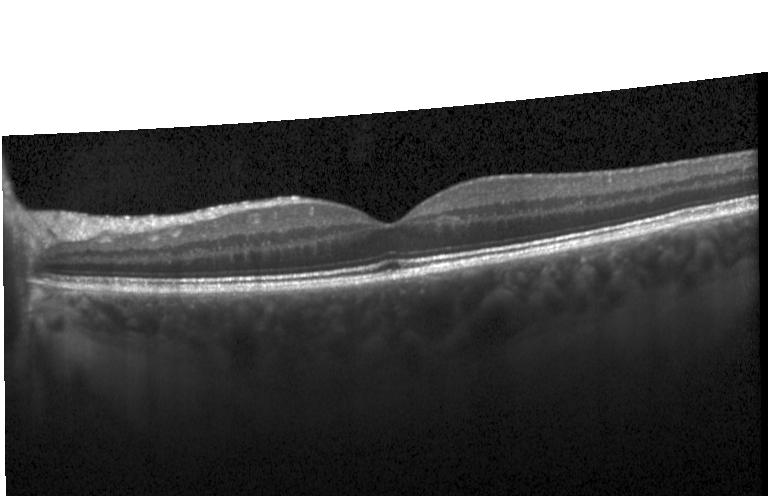

Spectral-domain OCT. Retinal OCT cross-section. Horizontal scan through the fovea — Diagnosis: no CNV, no DME, and no drusen.